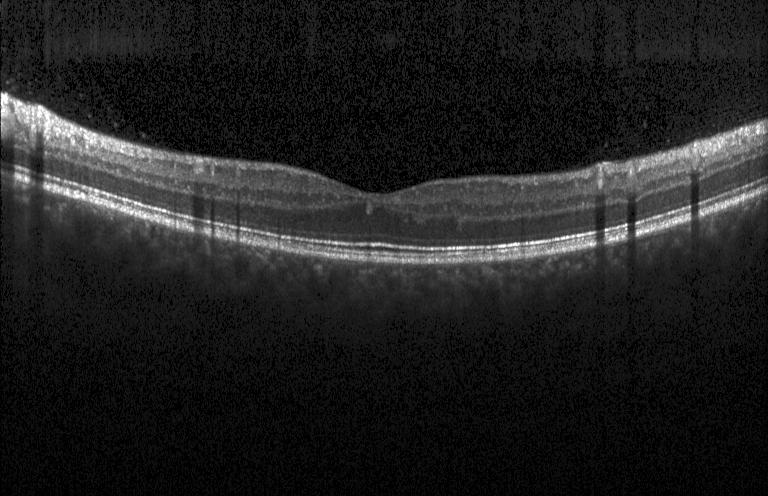

Horizontal scan through the fovea, retinal OCT B-scan
Macular OCT: no choroidal neovascularization, no diabetic macular edema, and no drusen.